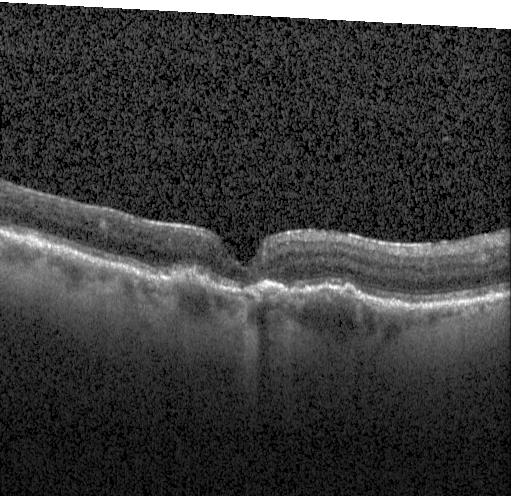

Through the macula, OCT B-scan, SD-OCT.
Finding: CNV.